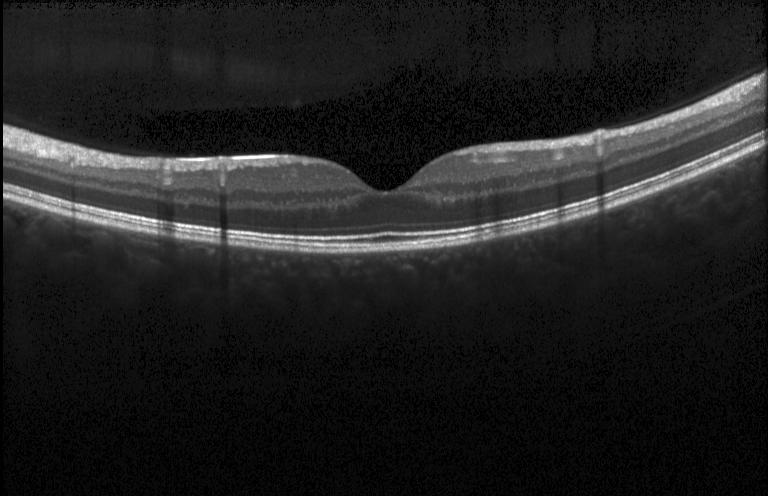 Spectral-domain OCT · instrument: Heidelberg Spectralis · retinal OCT cross-section · through the macula
OCT finding: neither choroidal neovascularization, diabetic macular edema, nor drusen.